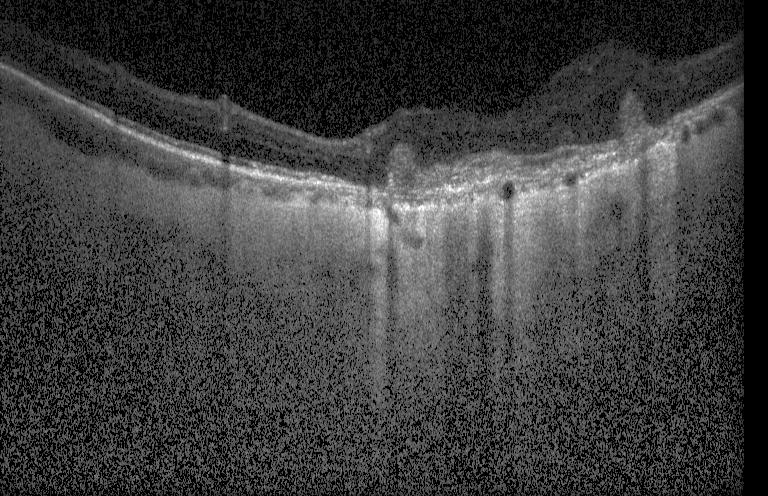

Spectral-domain optical coherence tomography · optical coherence tomography scan · acquired on a Heidelberg Spectralis.
Assessment: a choroidal neovascular membrane.